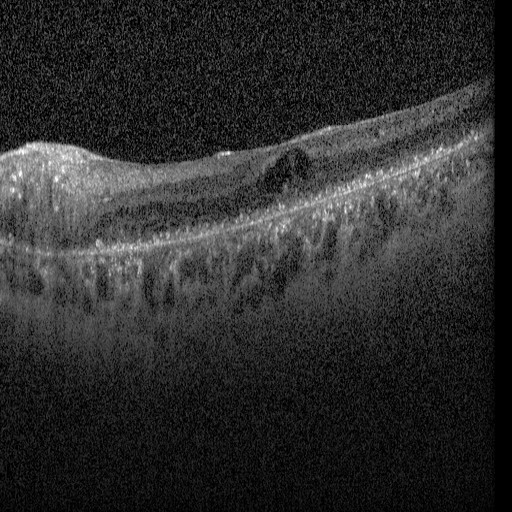
Retinal OCT B-scan
The scan shows diabetic macular edema.